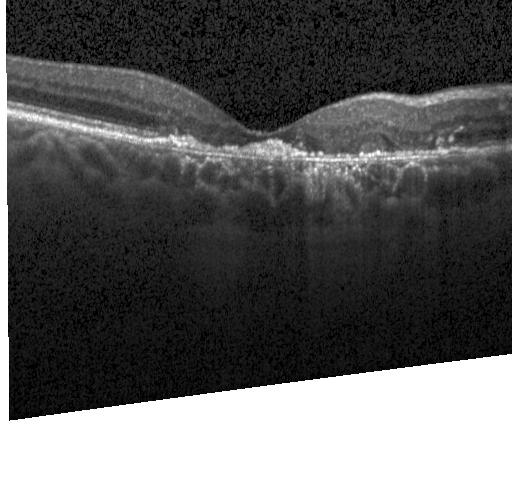

Finding: CNV.